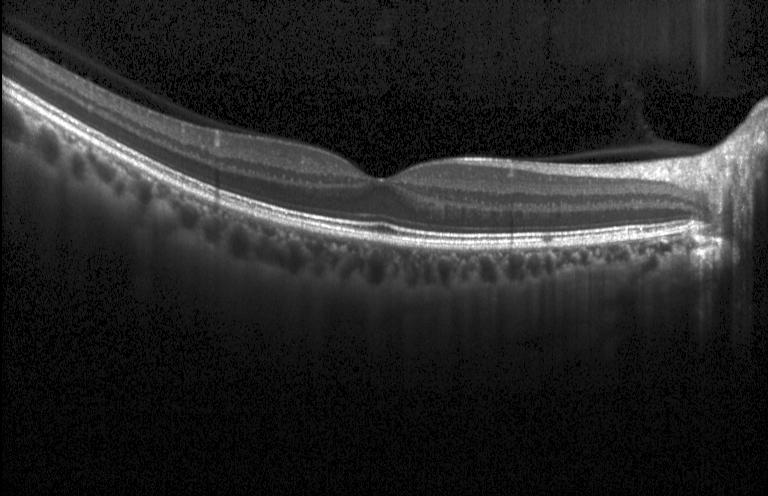

Impression: no CNV, no DME, and no drusen.